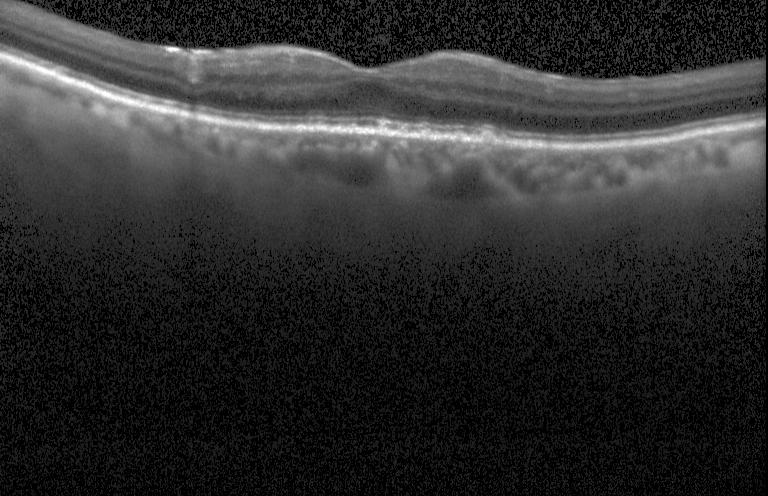 Macular scan; acquired on a Heidelberg Spectralis; optical coherence tomography scan. Diagnosis: multiple drusen.